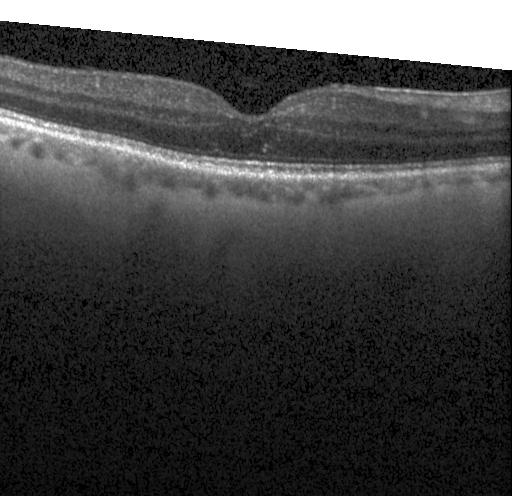
Retinal OCT cross-section. Spectral-domain optical coherence tomography — Assessment: no evidence of choroidal neovascularization, diabetic macular edema, or drusen.